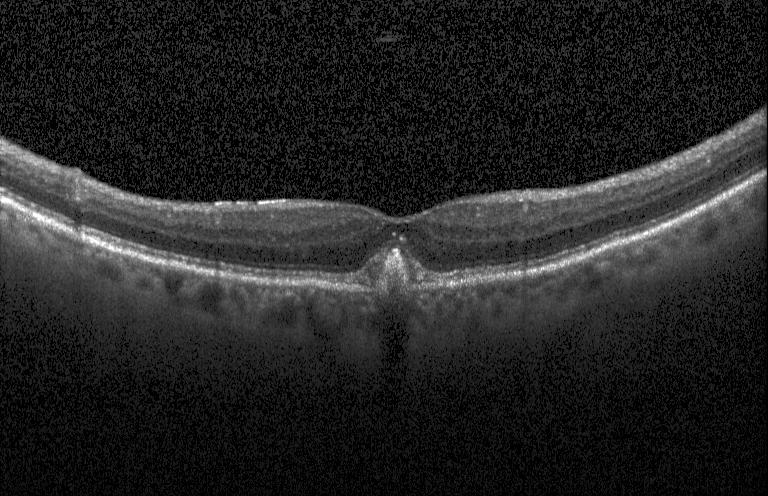
OCT line scan, macular scan, spectral-domain optical coherence tomography.
Assessment: choroidal neovascularization.